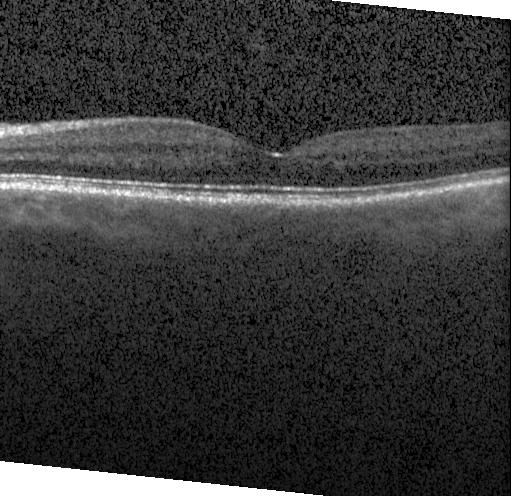
Macular scan, optical coherence tomography scan, Heidelberg Spectralis OCT system. Finding: neither choroidal neovascularization, diabetic macular edema, nor drusen.